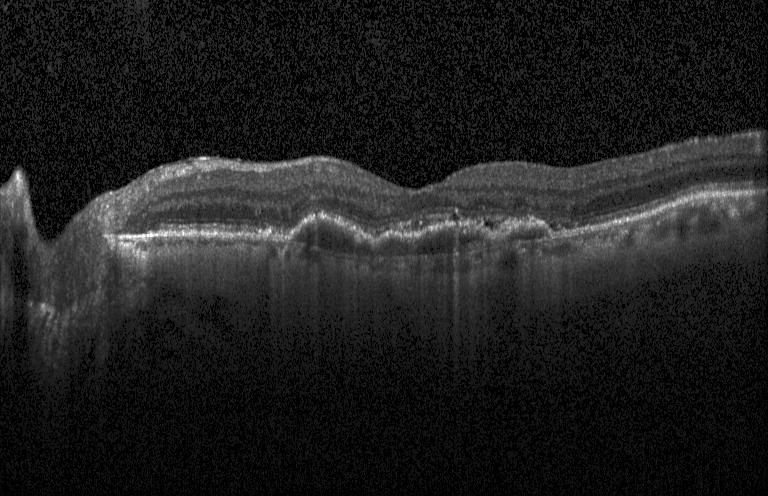
Assessment: choroidal neovascularization (CNV).